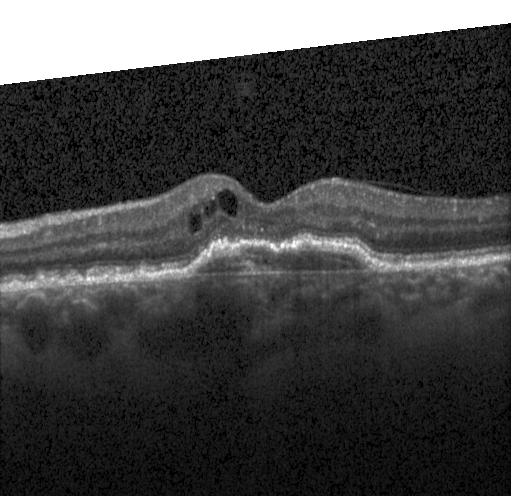

Dx: a choroidal neovascular membrane.